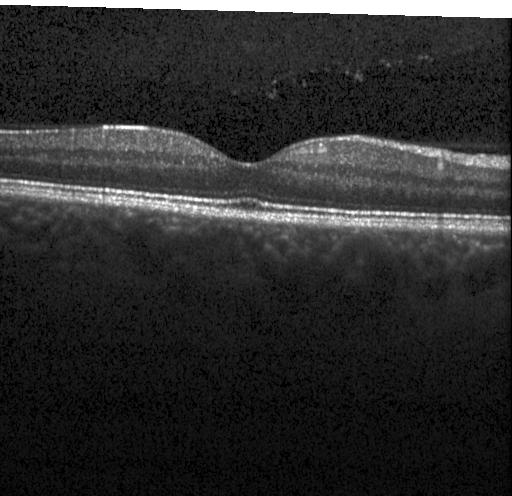 Retinal OCT B-scan
This B-scan demonstrates no CNV, no DME, and no drusen.